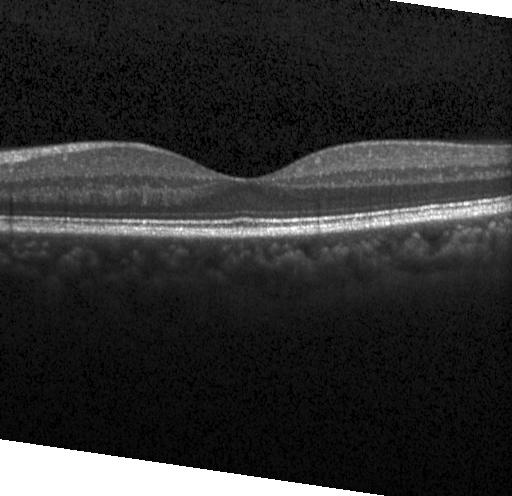 Spectral-domain OCT B-scan: no CNV, no DME, and no drusen.